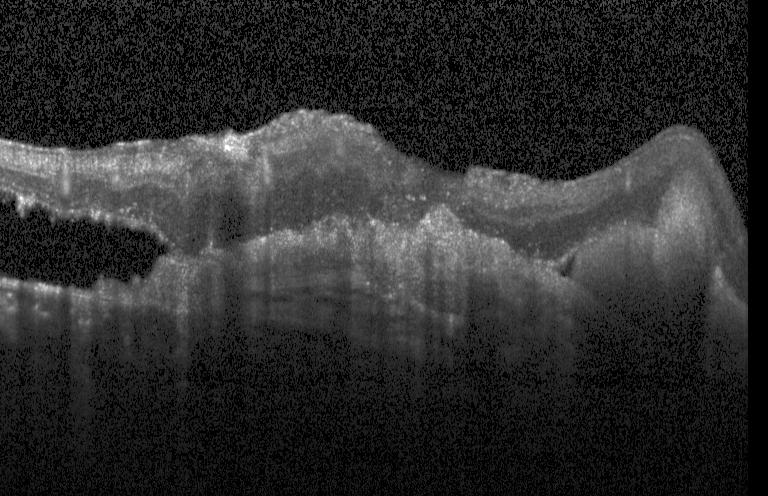
Assessment: CNV.